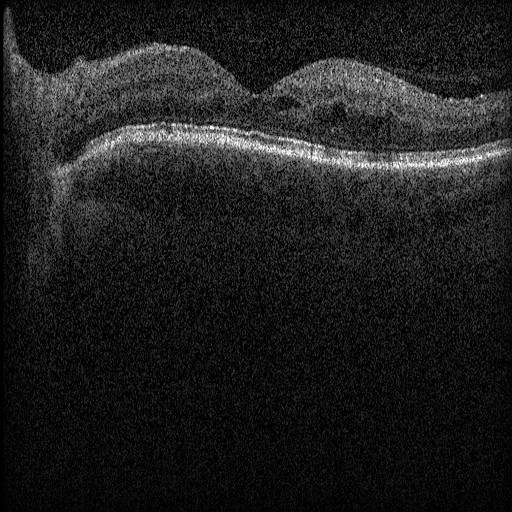 Retinal OCT B-scan
The scan shows DME.